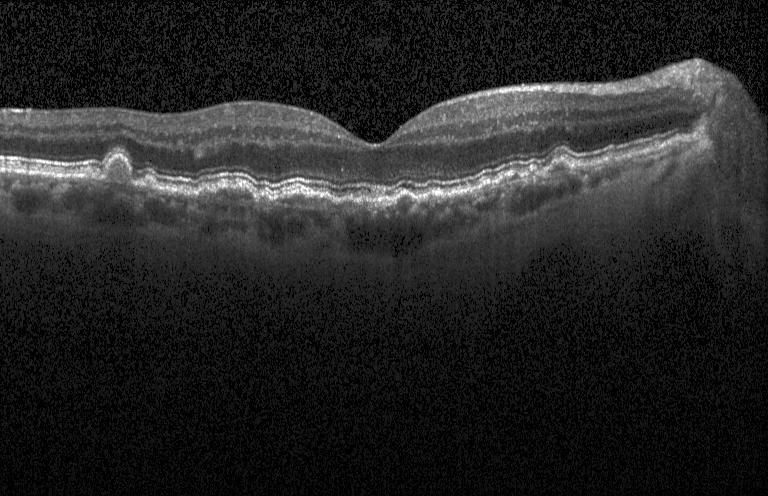

OCT B-scan. OCT finding: sub-RPE drusenoid deposits.